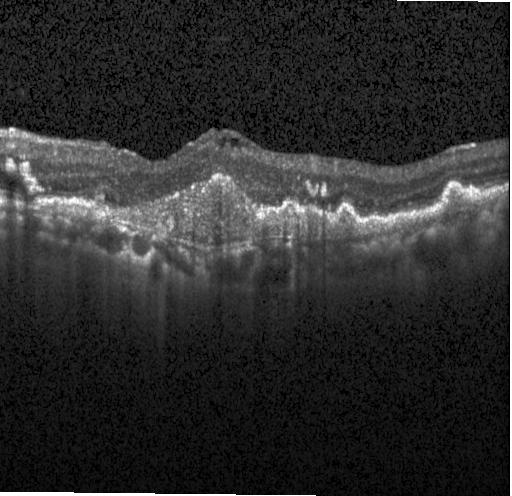
Dx: CNV.